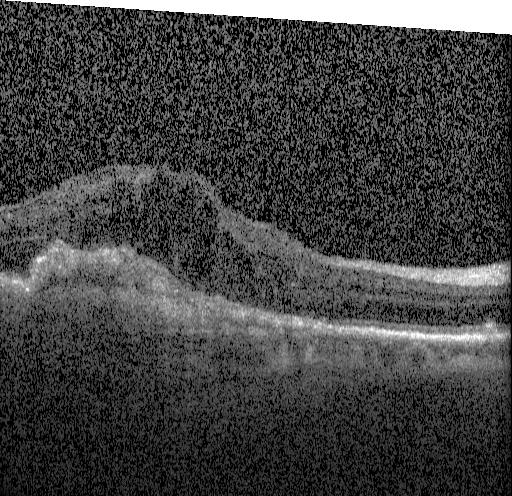 Spectral-domain optical coherence tomography. Optical coherence tomography B-scan. Macular OCT: choroidal neovascularization.